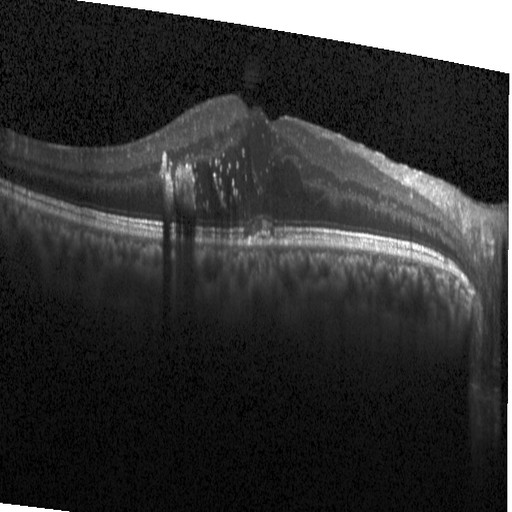
Retinal OCT B-scan; instrument: Heidelberg Spectralis — Diagnosis: diabetic macular edema (DME).